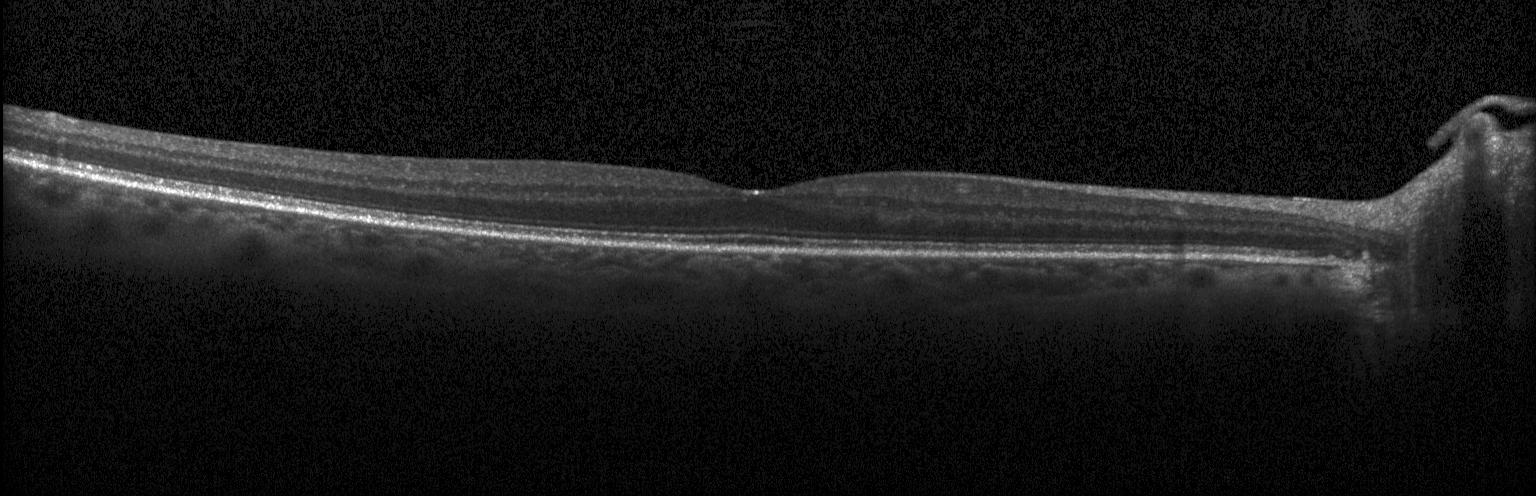
Through the macula · OCT line scan · SD-OCT
Assessment: no evidence of CNV, DME, or drusen.